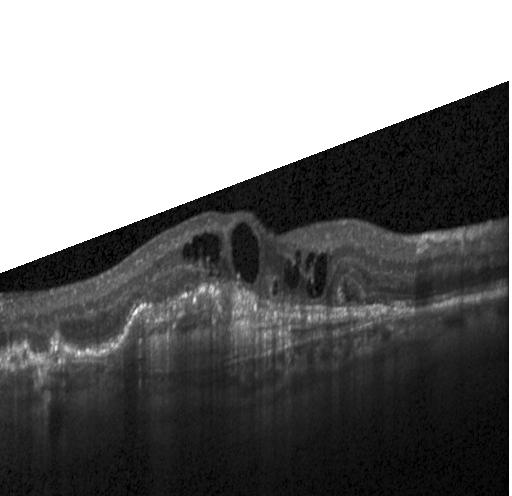 Finding: choroidal neovascularization.